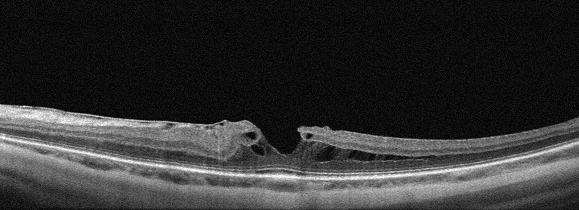

Optical coherence tomography scan; acquired on an Optovue Avanti RTVue XR; left eye
Finding: vitreomacular interface disease.